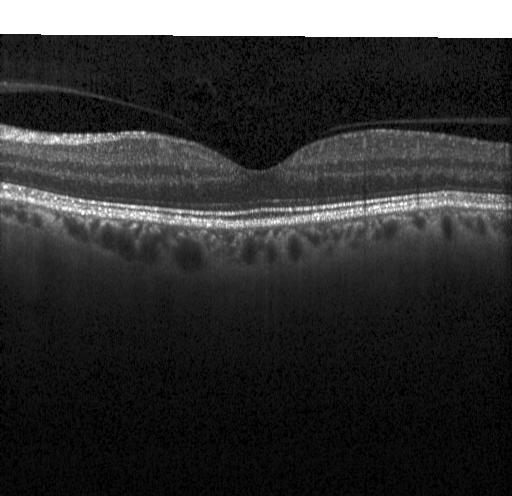

Retinal OCT B-scan
Assessment: no evidence of choroidal neovascularization, diabetic macular edema, or drusen.